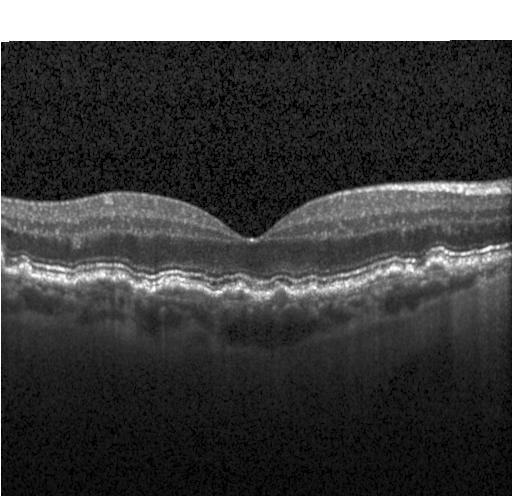
Instrument: Heidelberg Spectralis; spectral-domain OCT; fovea-centered; retinal OCT cross-section.
This B-scan demonstrates multiple drusen.